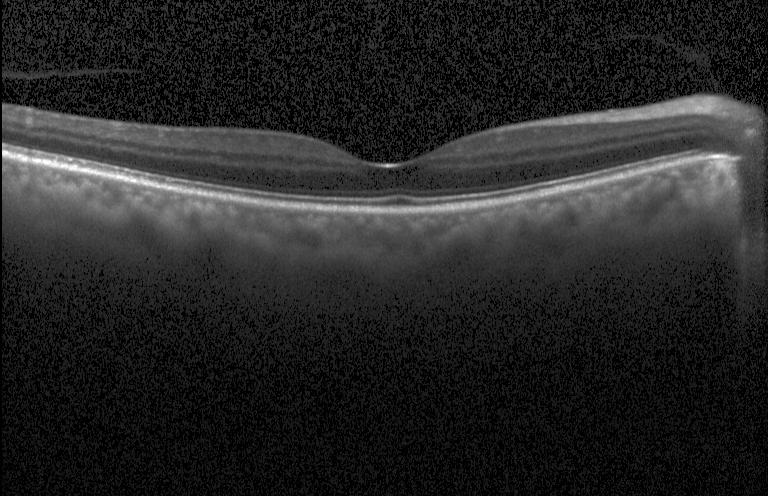
OCT B-scan showing no choroidal neovascularization, no diabetic macular edema, and no drusen.